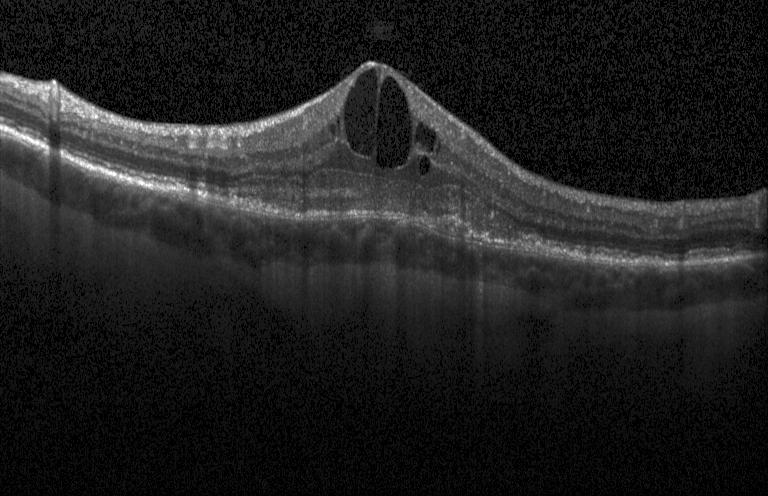
Diagnosis: choroidal neovascularization (CNV).